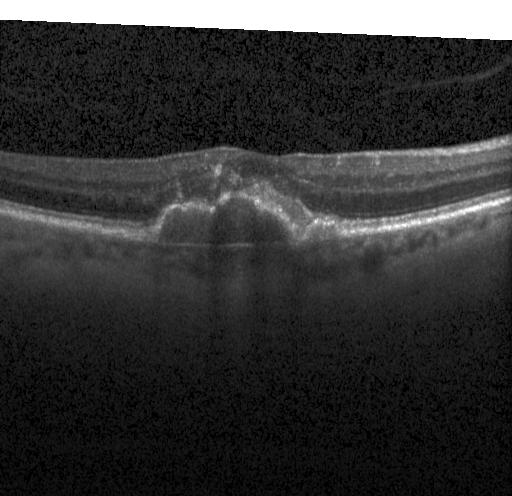 Horizontal scan through the fovea · SD-OCT · retinal OCT cross-section — Diagnosis: a choroidal neovascular membrane.